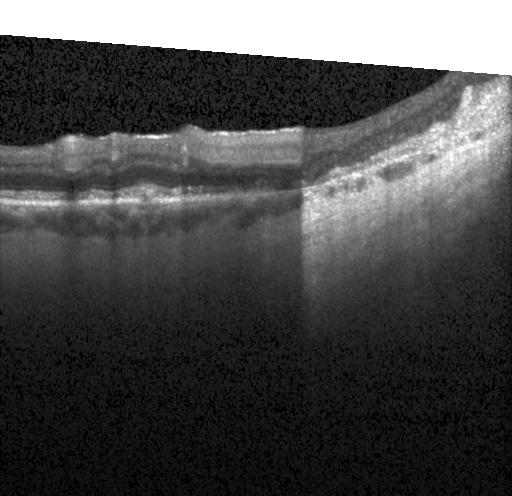

Optical coherence tomography B-scan · through the macula · spectral-domain OCT
This B-scan demonstrates choroidal neovascularization (CNV).